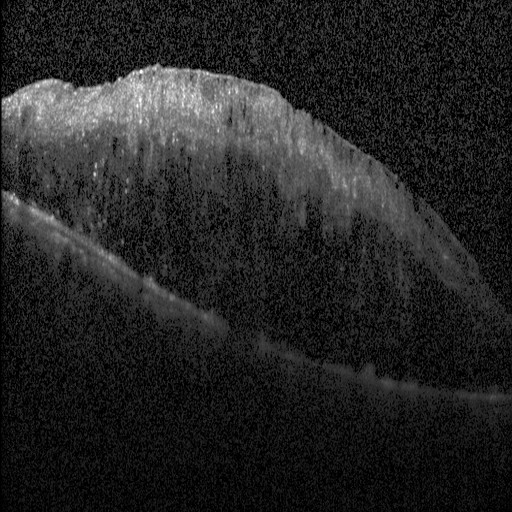
OCT line scan. Horizontal scan through the fovea. SD-OCT
Finding: diabetic macular edema.